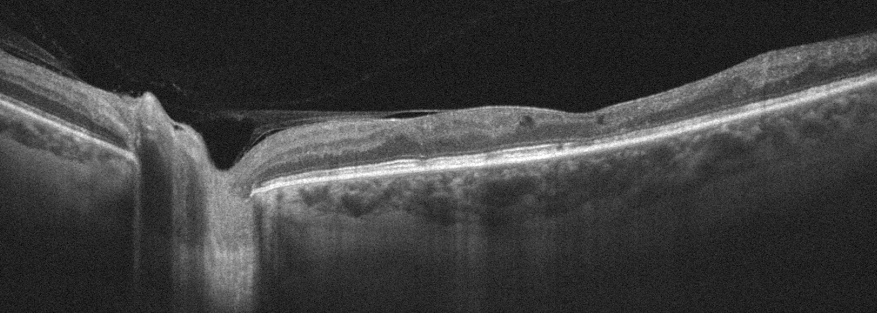
Through the macula · instrument: Optovue Avanti RTVue XR · retinal OCT B-scan. Diagnosis: DME.